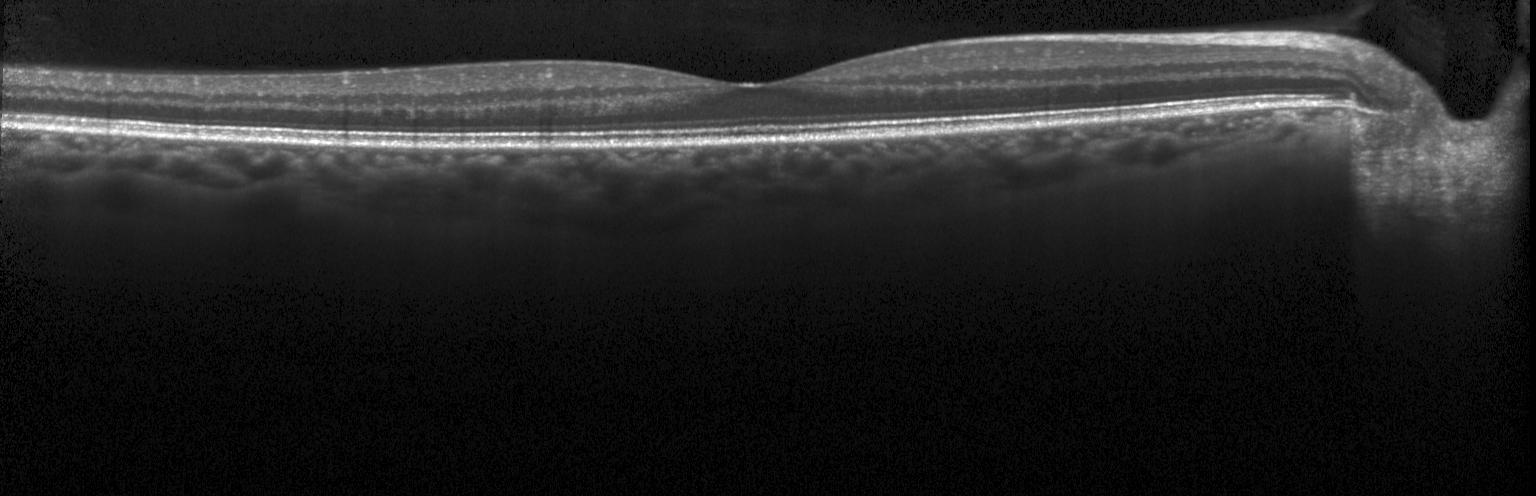

Retinal OCT cross-section · spectral-domain optical coherence tomography. OCT finding: no CNV, no DME, and no drusen.